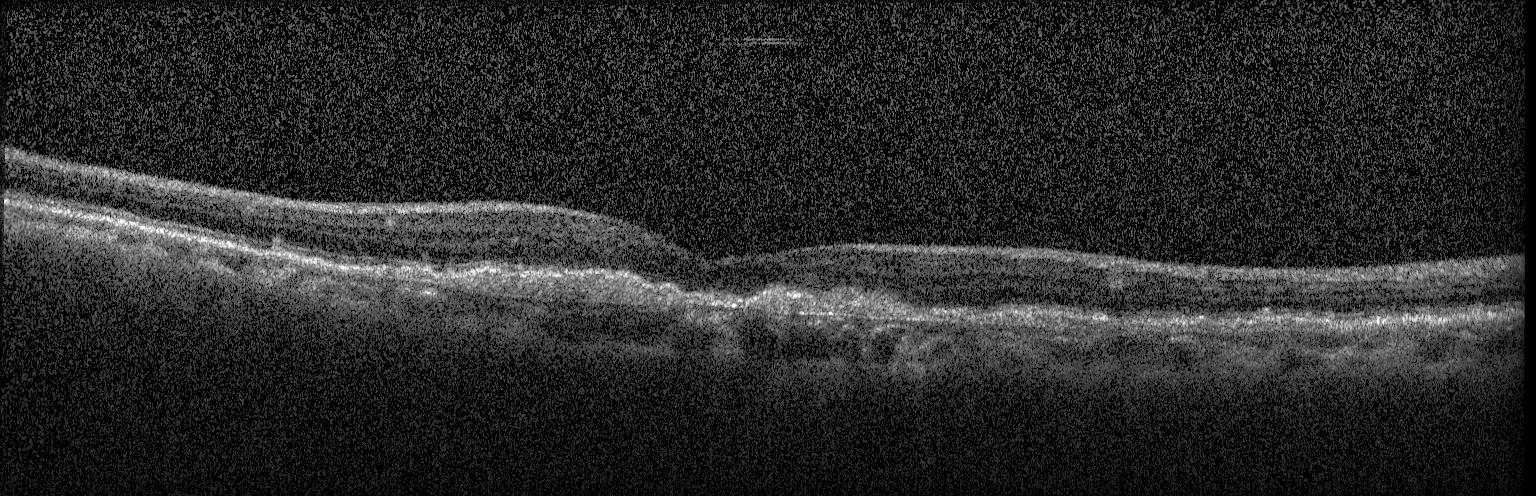
Retinal OCT cross-section; spectral-domain OCT
This B-scan demonstrates a choroidal neovascular membrane.